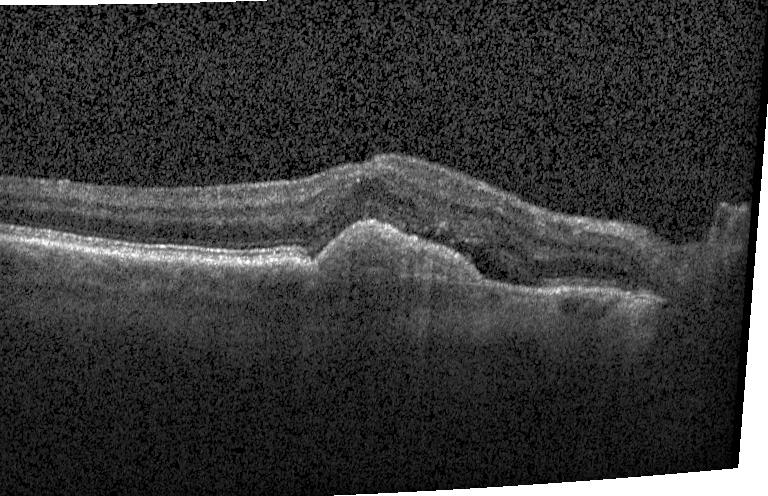

Heidelberg Spectralis, centered on the fovea, OCT B-scan, SD-OCT
Diagnosis: choroidal neovascularization.